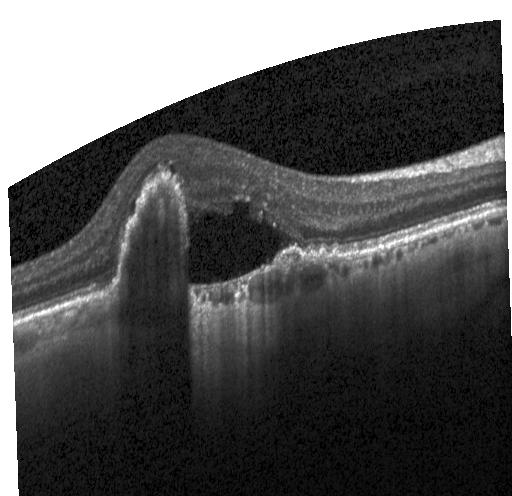 Optical coherence tomography scan · fovea-centered
Finding: CNV.